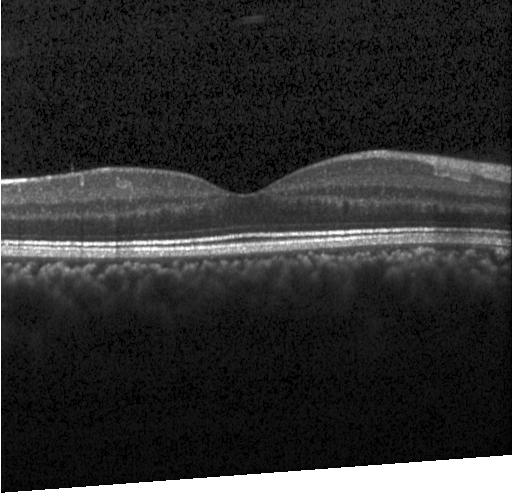

Through the macula · OCT line scan
Macular OCT: neither CNV, DME, nor drusen.